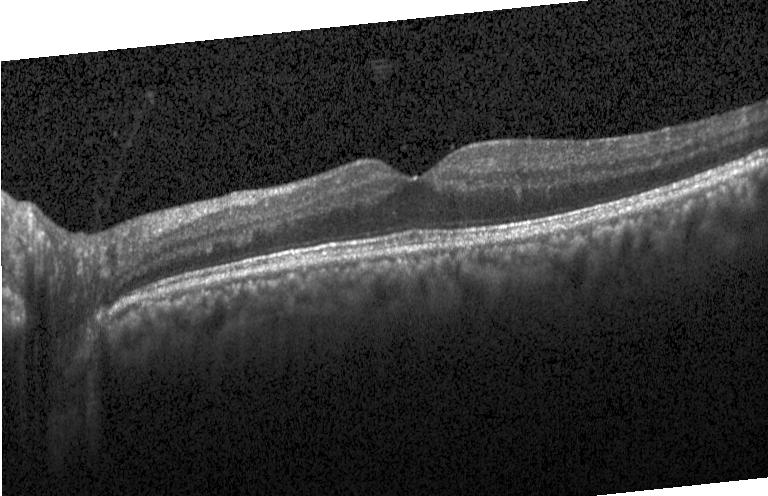
Spectral-domain OCT B-scan: no choroidal neovascularization, diabetic macular edema, or drusen.